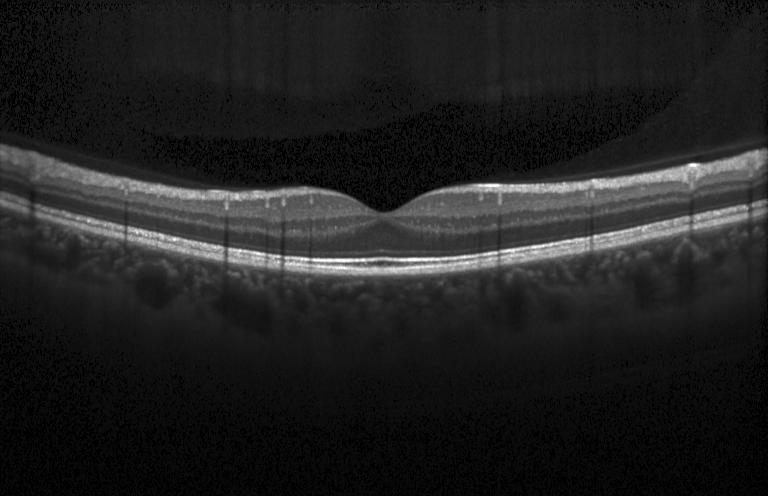
OCT finding: no choroidal neovascularization, diabetic macular edema, or drusen.